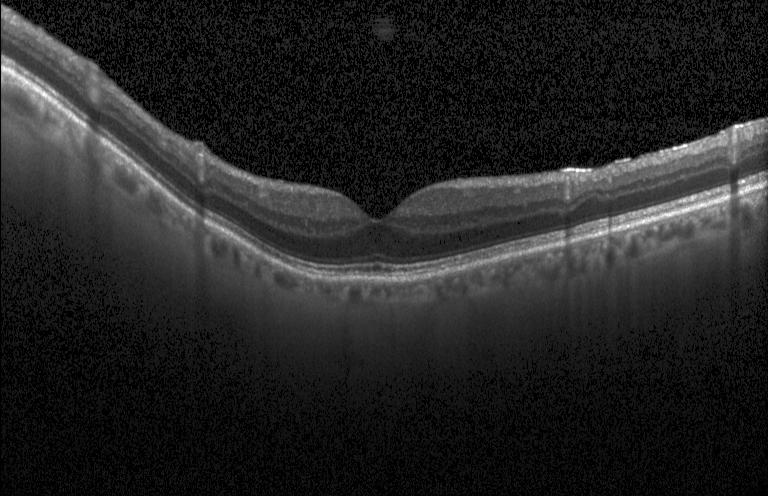
Diagnosis: no evidence of CNV, DME, or drusen.